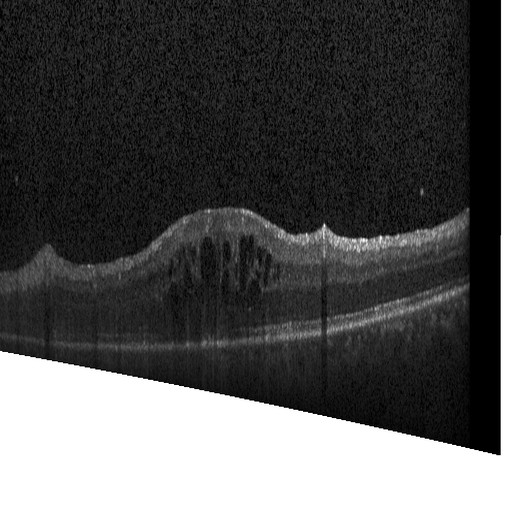

Centered on the fovea, optical coherence tomography B-scan — This B-scan demonstrates diabetic macular edema (DME).